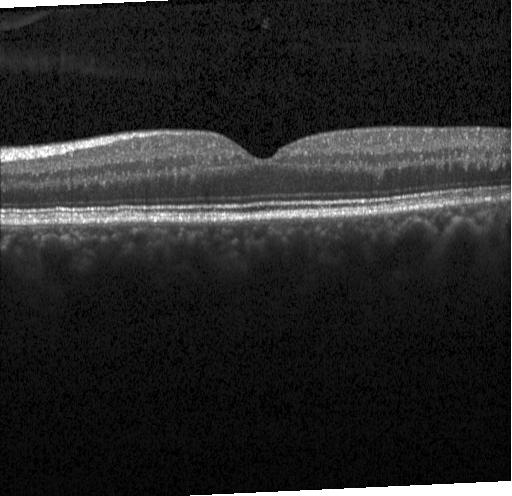

Retinal OCT cross-section — Dx: no choroidal neovascularization, diabetic macular edema, or drusen.